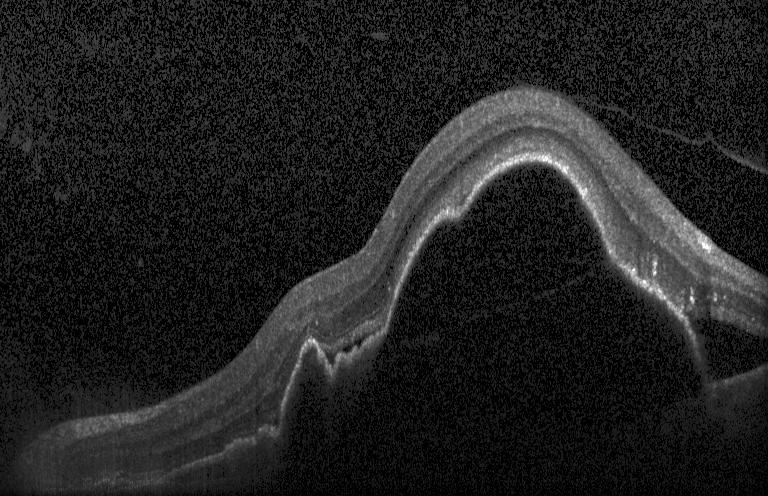
Retinal OCT B-scan. A choroidal neovascular membrane.